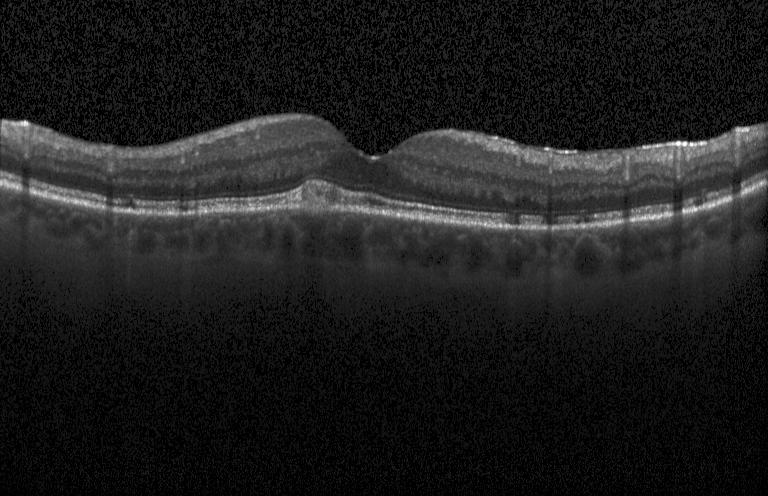

Through the macula, instrument: Heidelberg Spectralis, SD-OCT, OCT B-scan. This B-scan demonstrates multiple drusen.